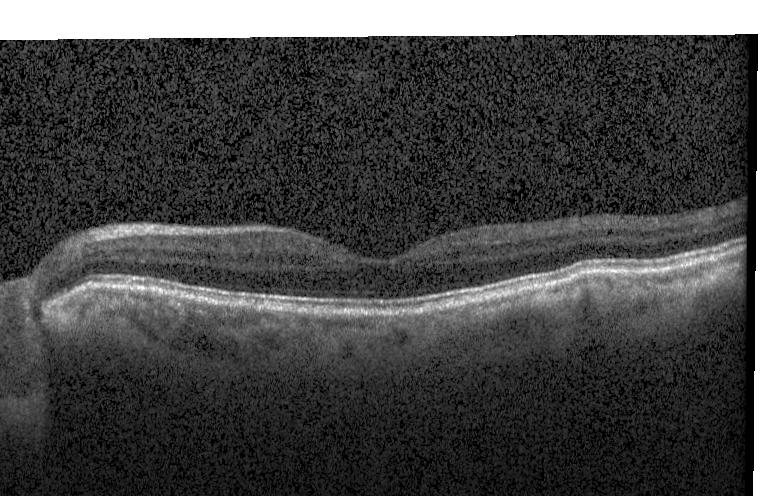

Retinal OCT B-scan; Heidelberg Spectralis OCT system; SD-OCT; macular scan. Impression: no choroidal neovascularization, diabetic macular edema, or drusen.